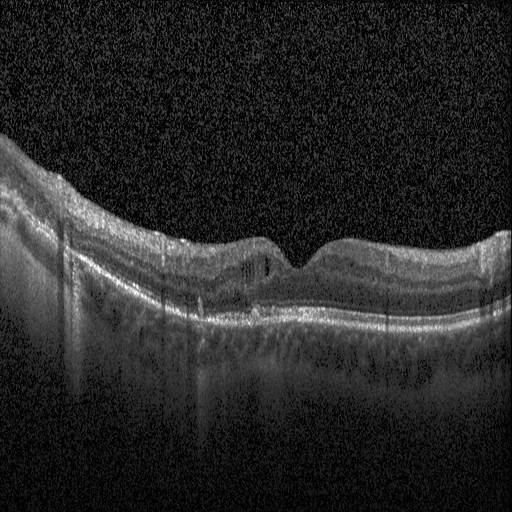
OCT B-scan showing DME.